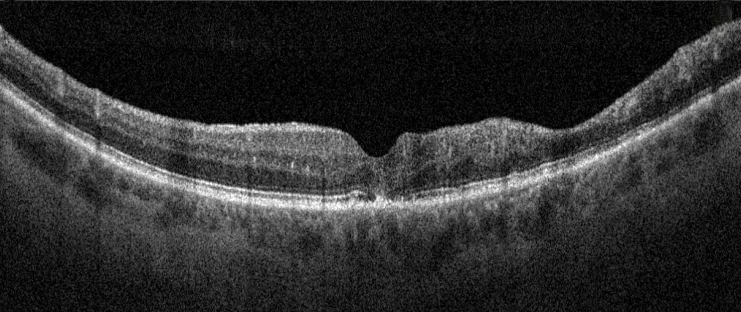 OCT B-scan showing diabetic macular edema (DME).